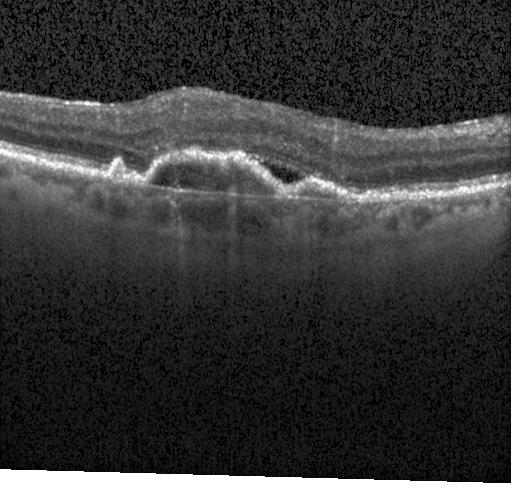 Heidelberg Spectralis; optical coherence tomography scan; spectral-domain optical coherence tomography — Impression: a choroidal neovascular membrane.